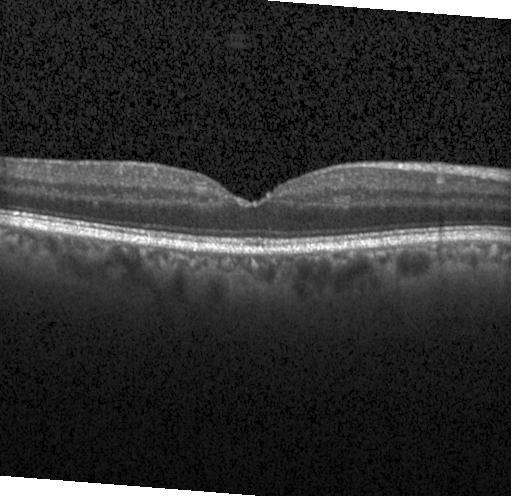 Instrument: Heidelberg Spectralis, OCT line scan, centered on the fovea, spectral-domain optical coherence tomography — This B-scan demonstrates no choroidal neovascularization, no diabetic macular edema, and no drusen.